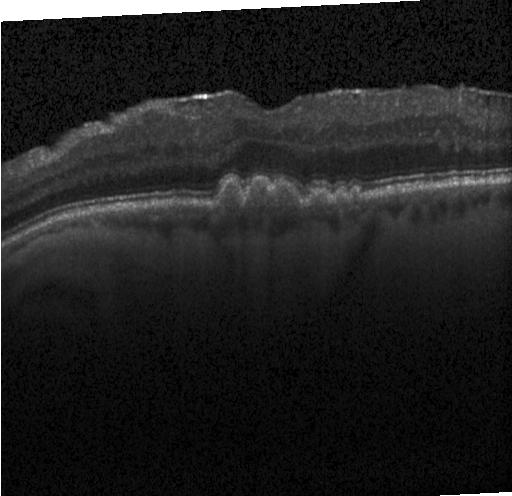 Heidelberg Spectralis OCT system, OCT line scan, SD-OCT
Diagnosis: multiple drusen.